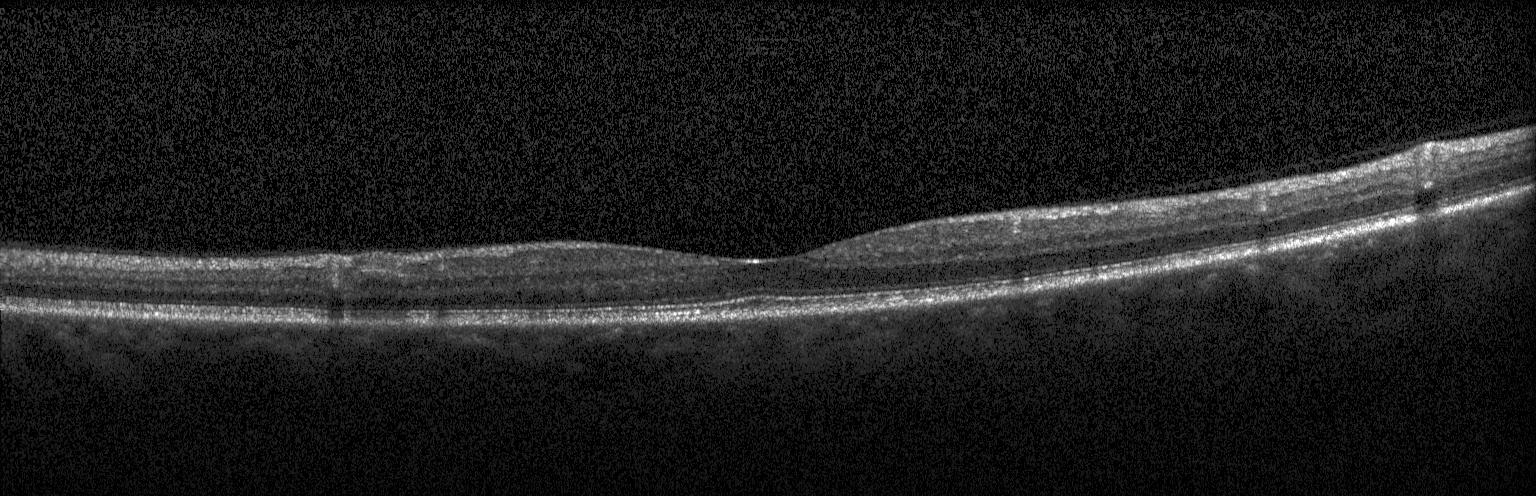 Diagnosis: no CNV, no DME, and no drusen.